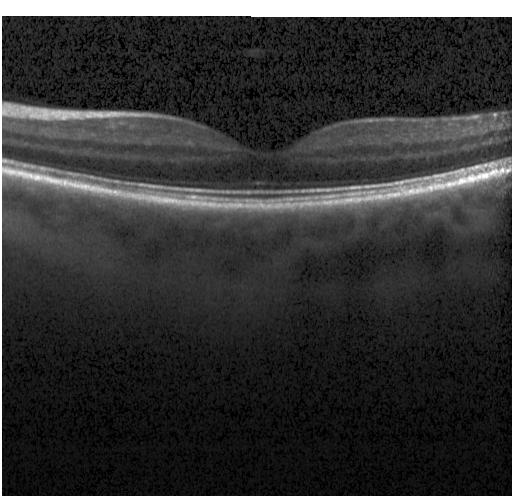
No CNV, DME, or drusen.